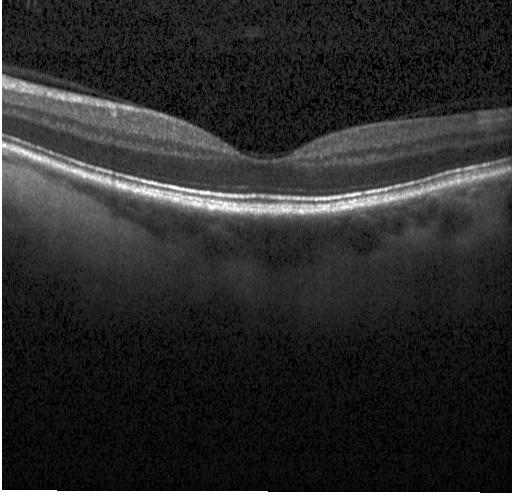 Acquired on a Heidelberg Spectralis, spectral-domain OCT, optical coherence tomography scan. Impression: no evidence of choroidal neovascularization, diabetic macular edema, or drusen.